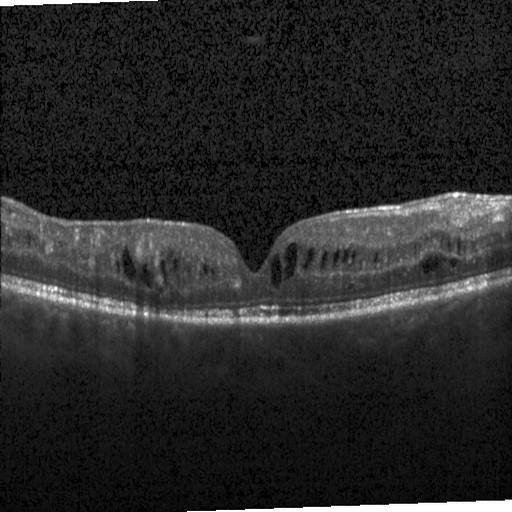

Impression: DME.